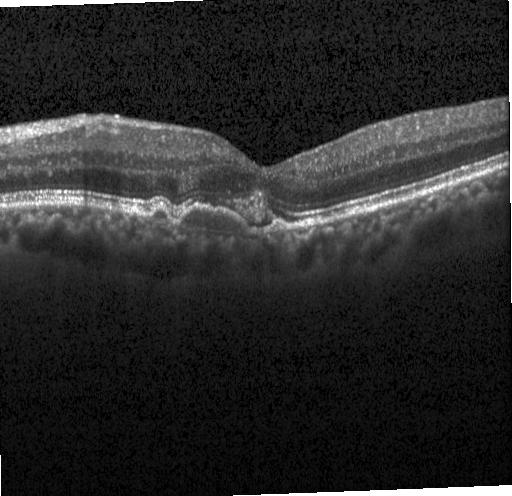
OCT B-scan
Diagnosis: choroidal neovascularization.